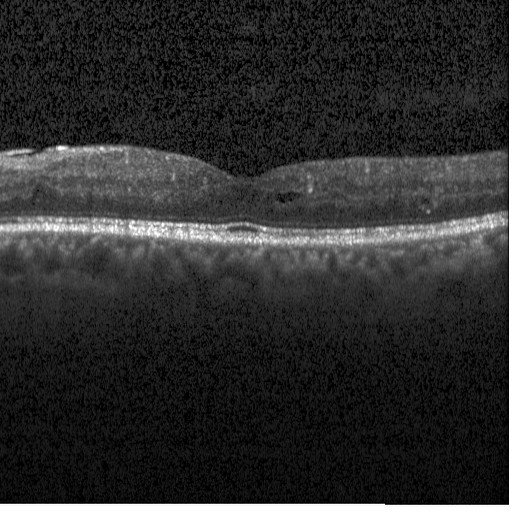
Retinal OCT cross-section
Assessment: diabetic macular edema.